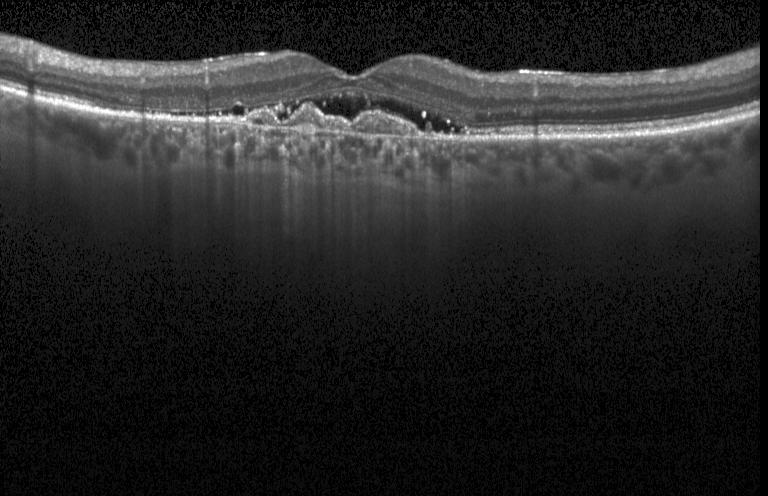

Heidelberg Spectralis. Fovea-centered. Retinal OCT cross-section. Impression: a choroidal neovascular membrane.